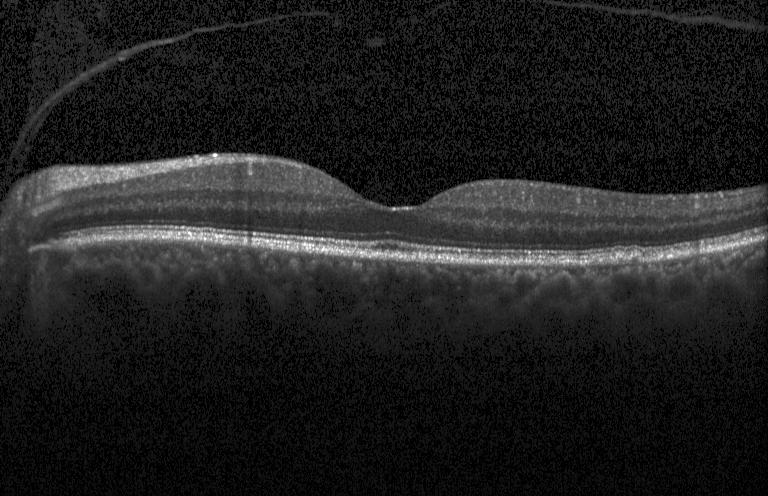

OCT line scan; centered on the fovea — Finding: no CNV, DME, or drusen.